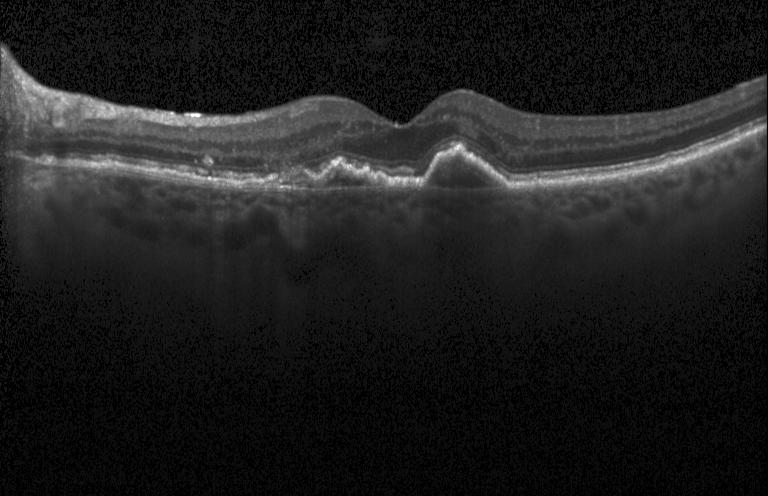 This B-scan demonstrates a choroidal neovascular membrane.